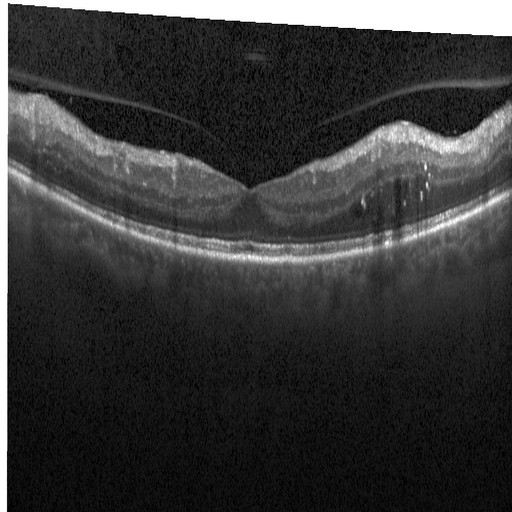 Acquired on a Heidelberg Spectralis · macular scan · OCT B-scan
Impression: diabetic macular edema.